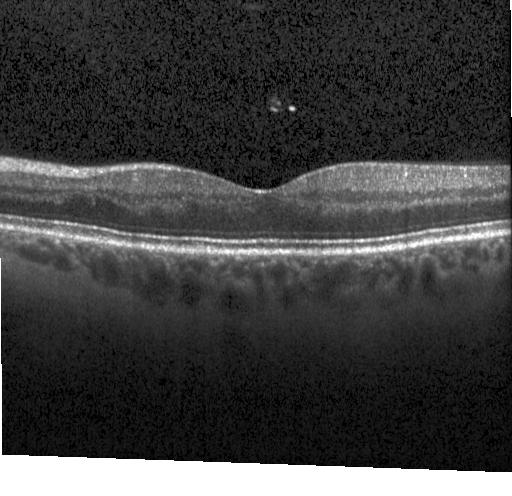

Finding: no choroidal neovascularization, diabetic macular edema, or drusen.